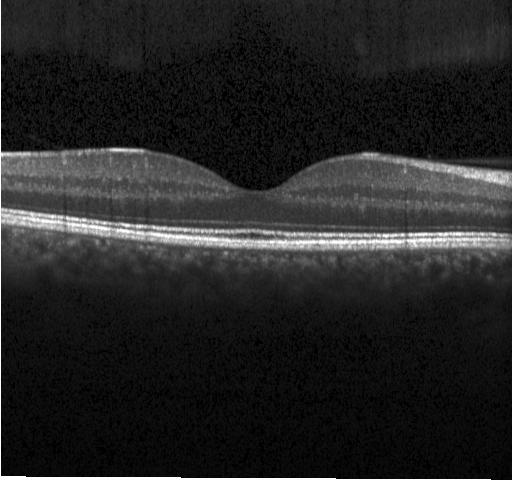
Fovea-centered · OCT line scan — The scan shows neither choroidal neovascularization, diabetic macular edema, nor drusen.